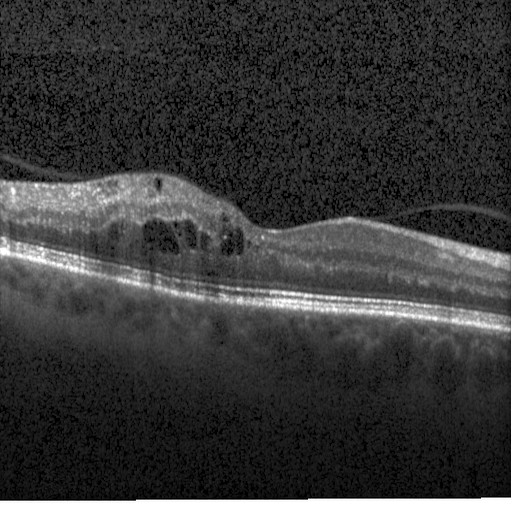
Spectral-domain OCT B-scan: DME.